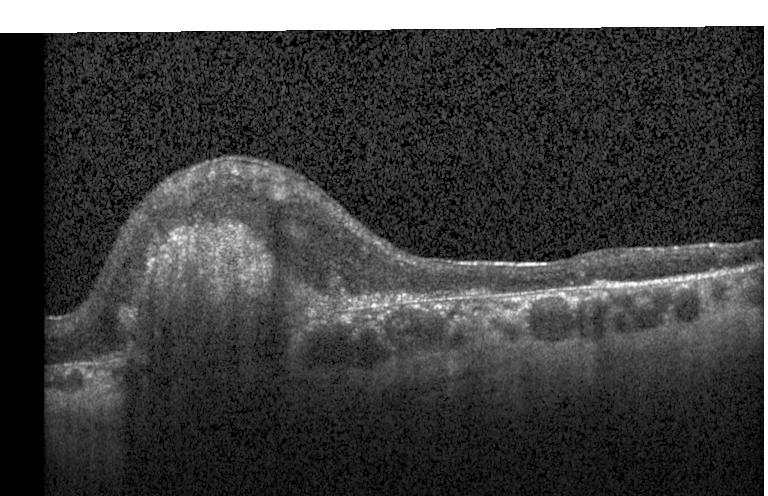

Retinal OCT cross-section showing a choroidal neovascular membrane.